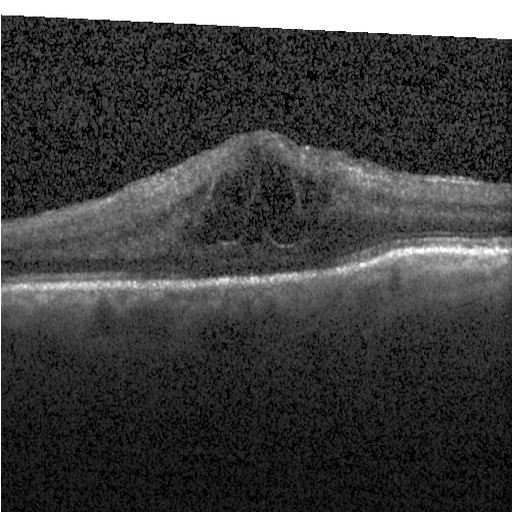
Heidelberg Spectralis OCT system; optical coherence tomography B-scan; macular scan
Finding: diabetic macular edema.